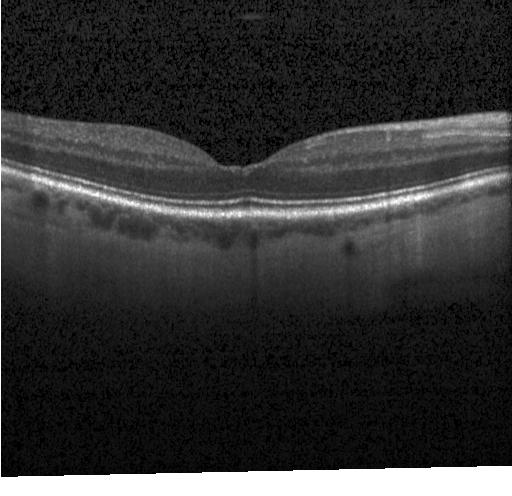
Macular OCT: no evidence of choroidal neovascularization, diabetic macular edema, or drusen.